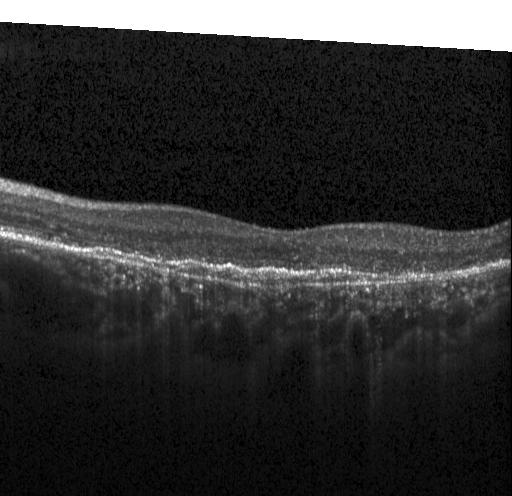 OCT scan showing a choroidal neovascular membrane.